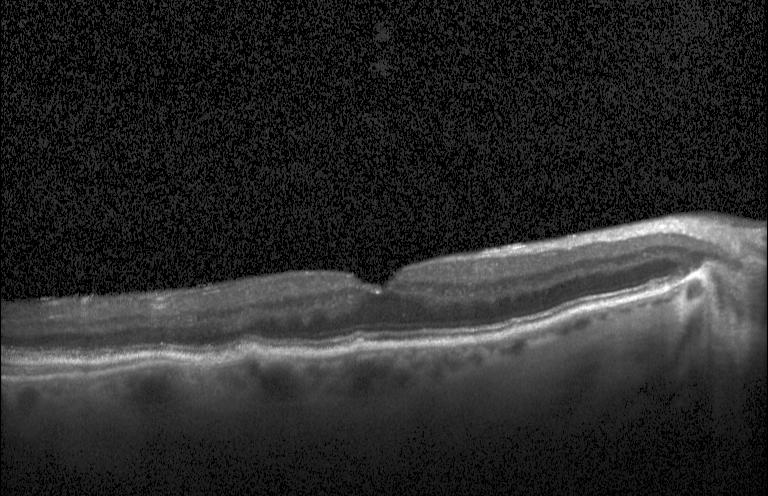

A choroidal neovascular membrane.